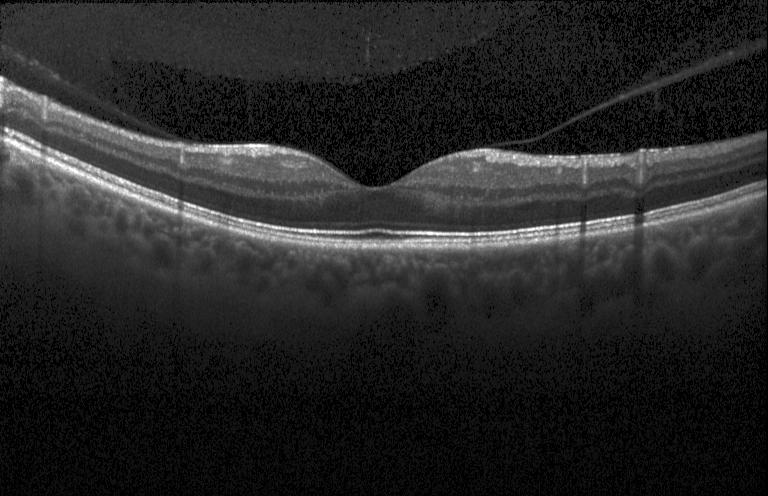 OCT line scan; spectral-domain optical coherence tomography; fovea-centered; Heidelberg Spectralis — This B-scan demonstrates no choroidal neovascularization, no diabetic macular edema, and no drusen.